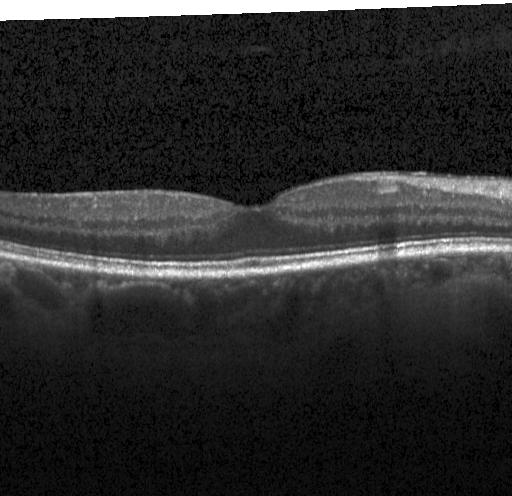

Heidelberg Spectralis, OCT line scan, through the macula, SD-OCT
Dx: no evidence of CNV, DME, or drusen.